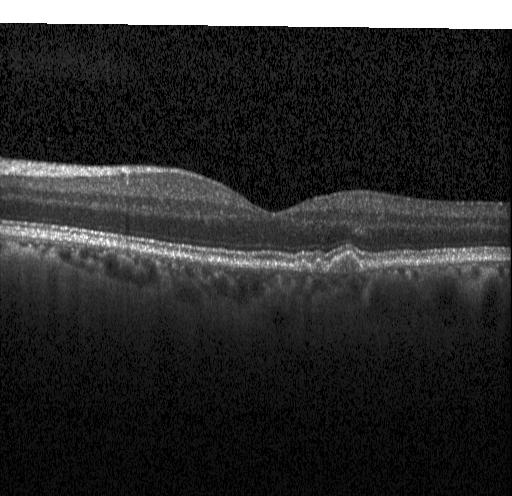

Dx: sub-RPE drusenoid deposits.